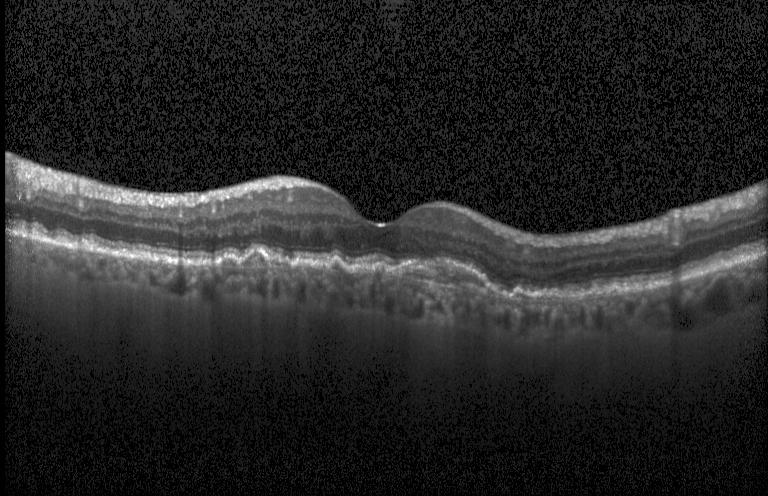 Optical coherence tomography B-scan; spectral-domain OCT
Assessment: a choroidal neovascular membrane.